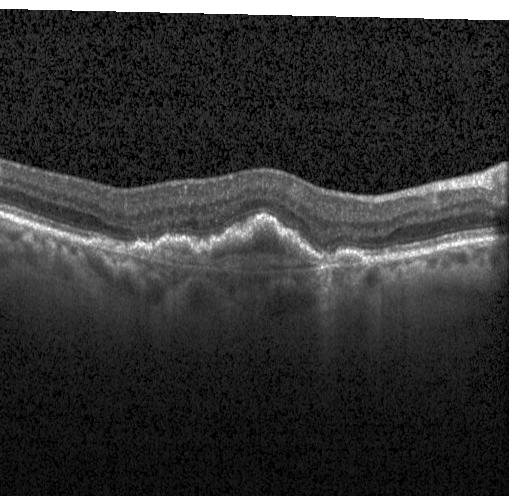

OCT scan showing choroidal neovascularization (CNV).